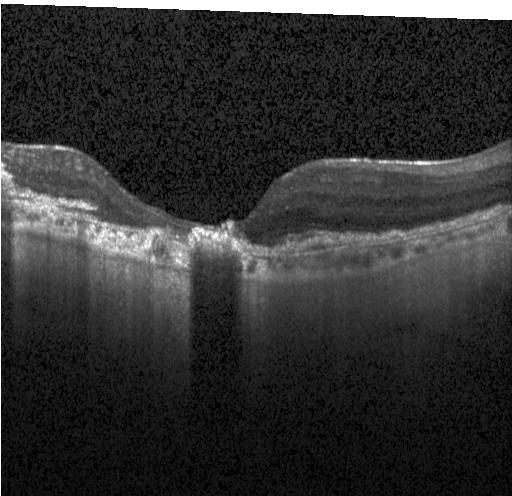
SD-OCT; OCT line scan.
CNV.